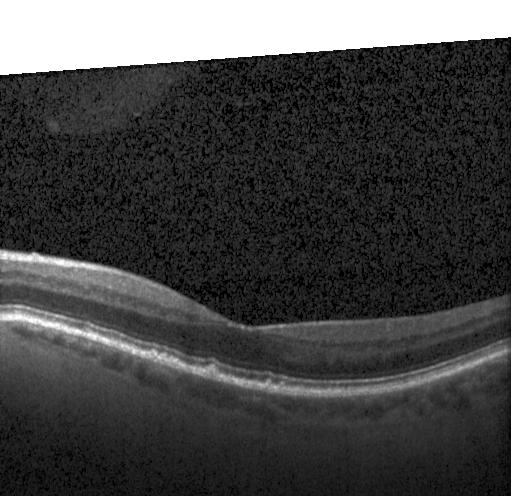 OCT scan showing drusen.